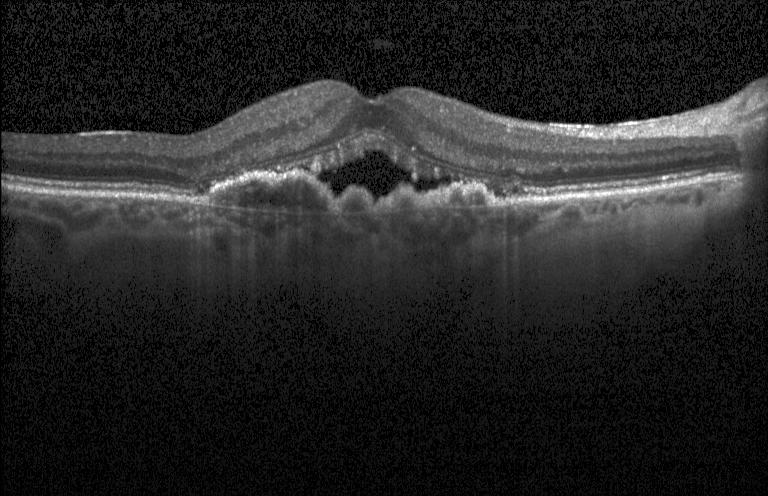

Impression: choroidal neovascularization.